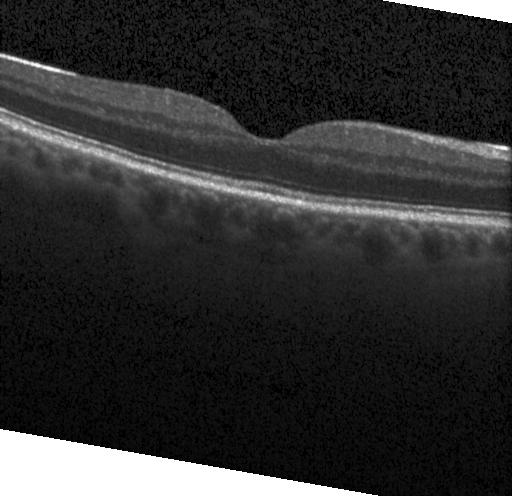

Macular OCT demonstrating no choroidal neovascularization, diabetic macular edema, or drusen.